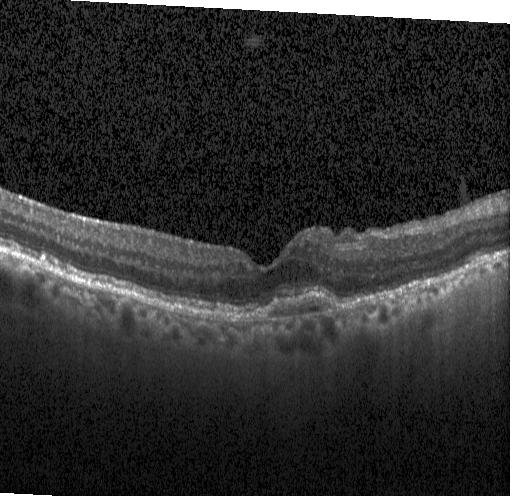 Optical coherence tomography B-scan
Impression: choroidal neovascularization (CNV).